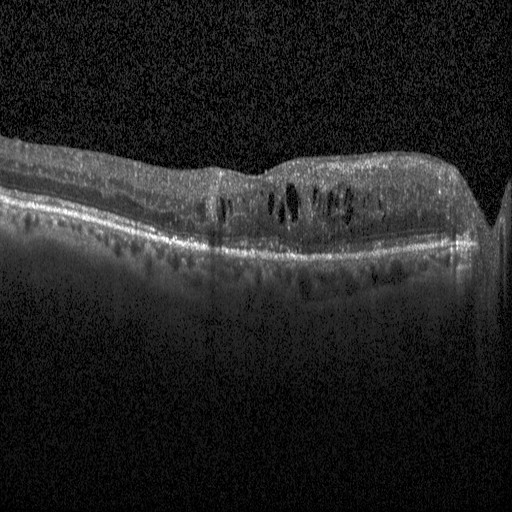
This B-scan demonstrates DME.